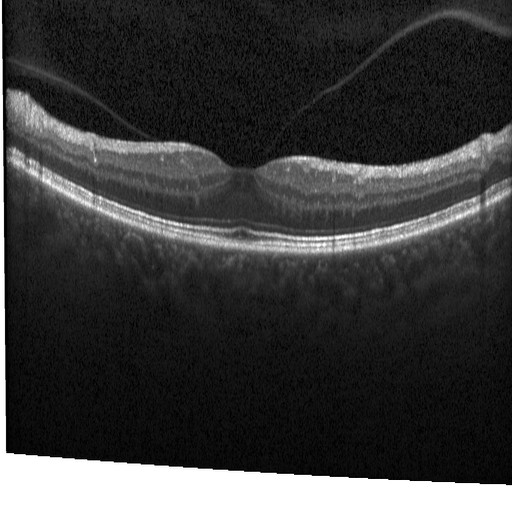 Retinal OCT B-scan. Spectral-domain OCT. Diagnosis: diabetic macular edema (DME).